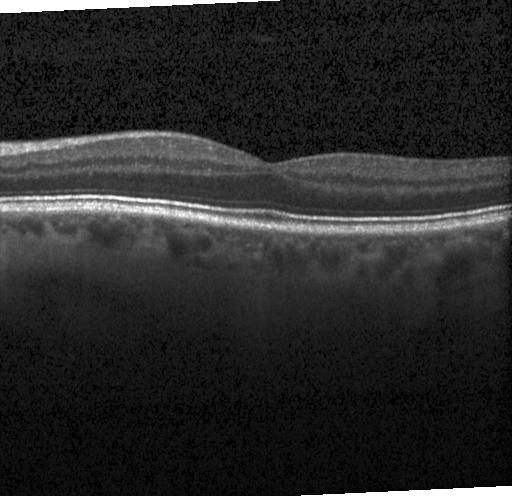

This B-scan demonstrates no evidence of choroidal neovascularization, diabetic macular edema, or drusen.